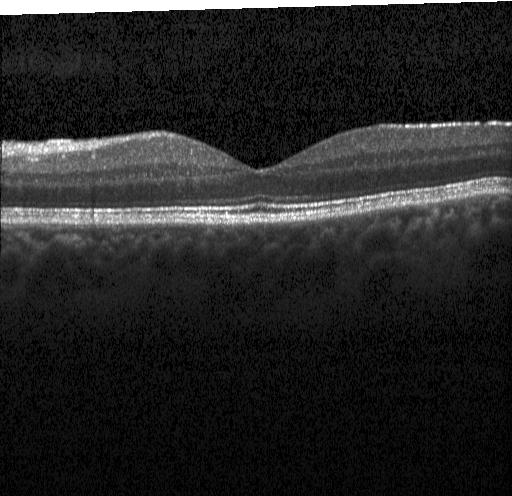

OCT B-scan; spectral-domain OCT. Dx: no CNV, DME, or drusen.